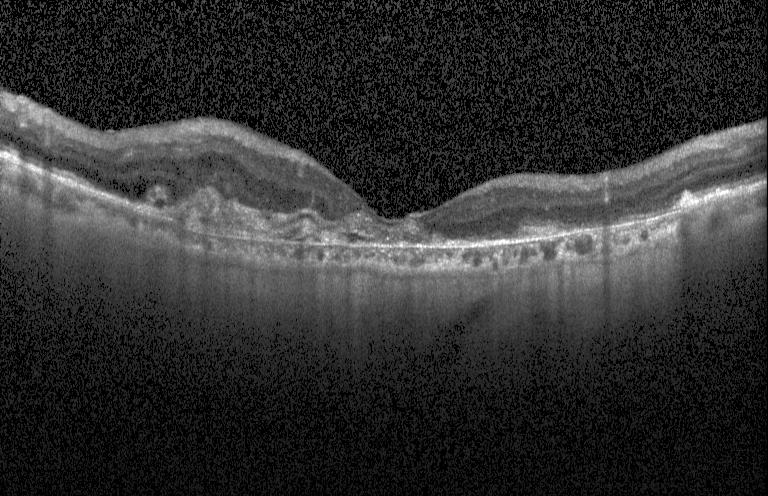

Diagnosis: choroidal neovascularization.